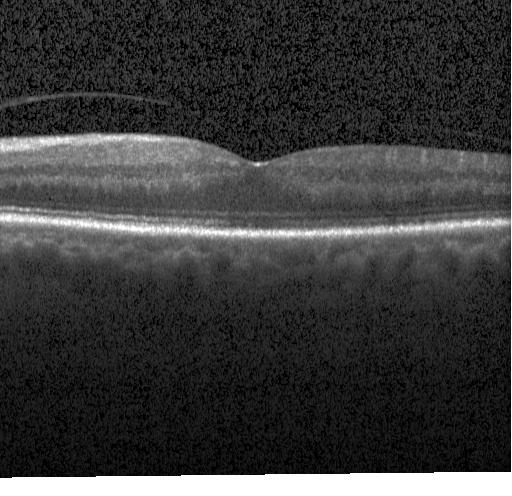

Retinal OCT B-scan · Heidelberg Spectralis OCT system
Diagnosis: no choroidal neovascularization, diabetic macular edema, or drusen.